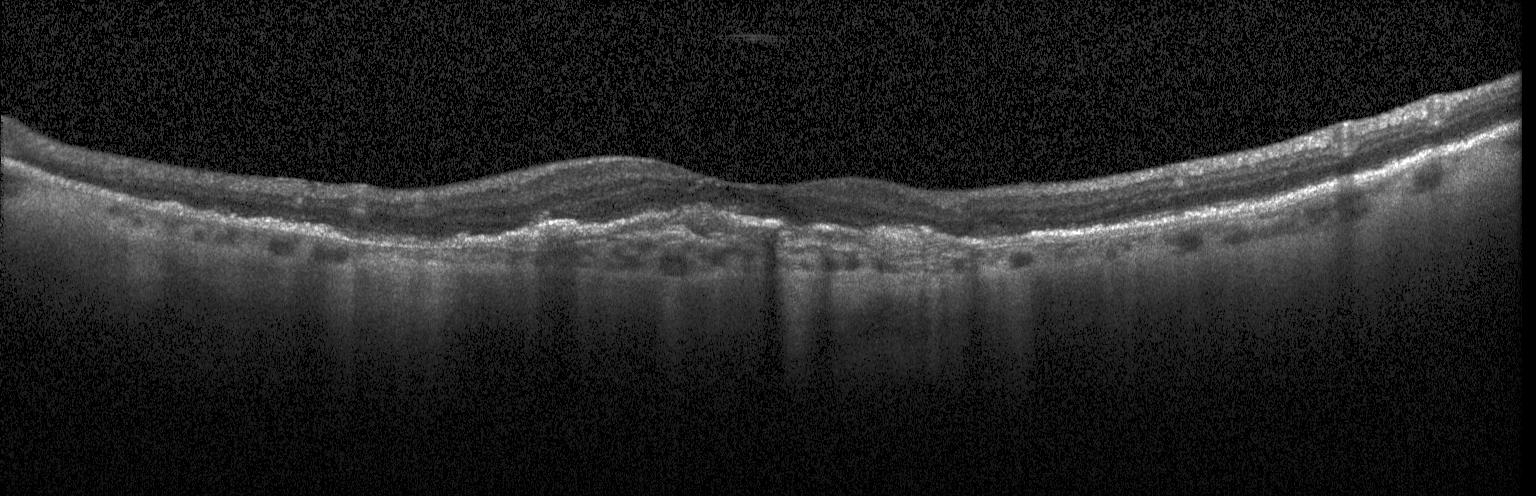 Macular OCT demonstrating CNV.